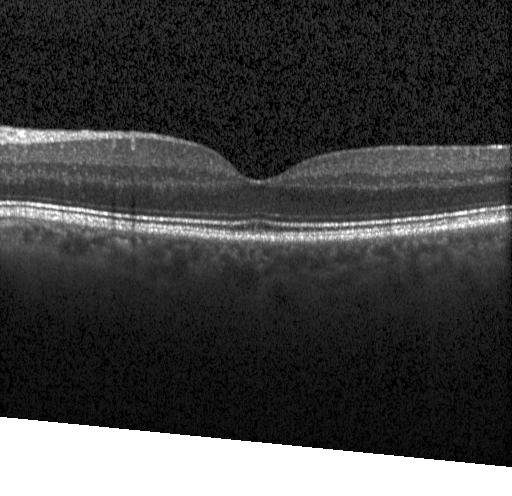 Retinal OCT B-scan — Finding: neither choroidal neovascularization, diabetic macular edema, nor drusen.